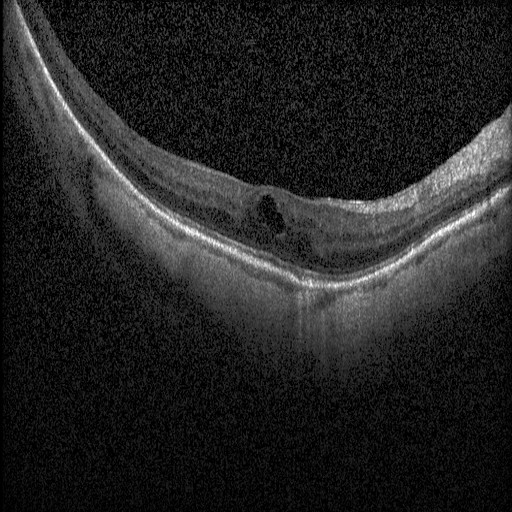 OCT B-scan
Finding: diabetic macular edema (DME).